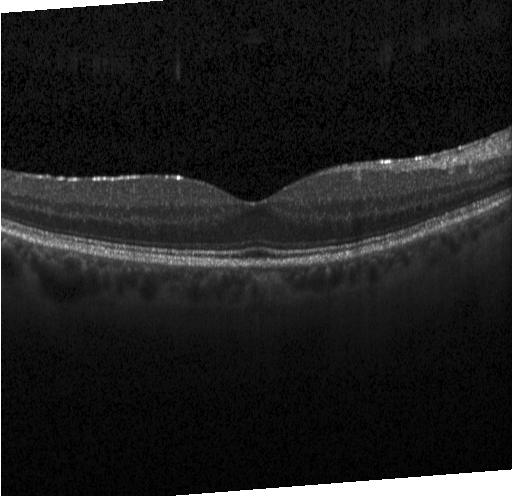
Diagnosis: no evidence of choroidal neovascularization, diabetic macular edema, or drusen.